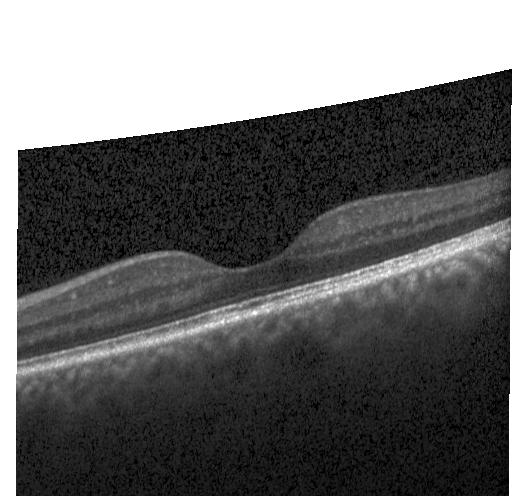 Macular scan · retinal OCT cross-section.
Finding: no choroidal neovascularization, no diabetic macular edema, and no drusen.